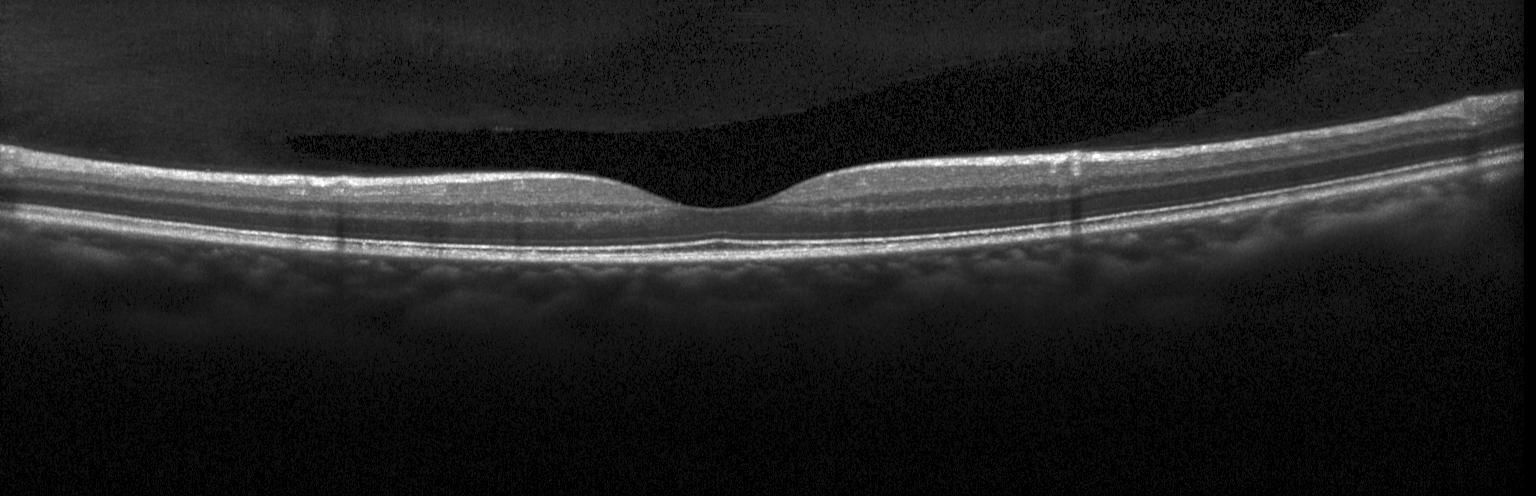
OCT B-scan
No CNV, DME, or drusen.